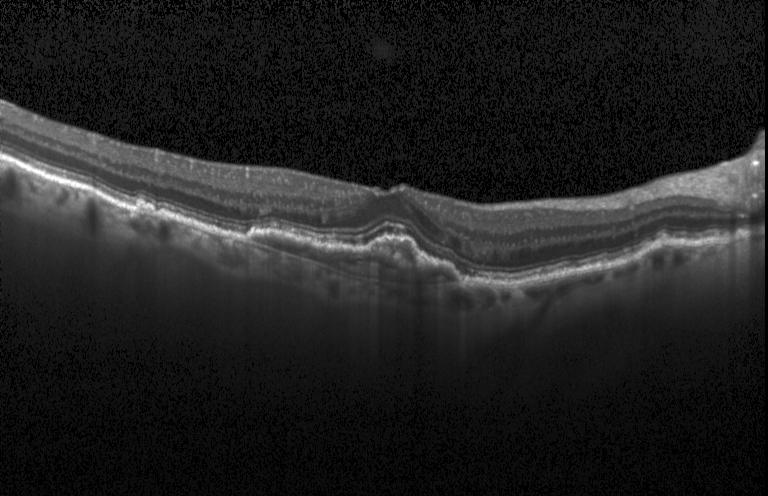
OCT line scan, fovea-centered, Heidelberg Spectralis. Diagnosis: a choroidal neovascular membrane.